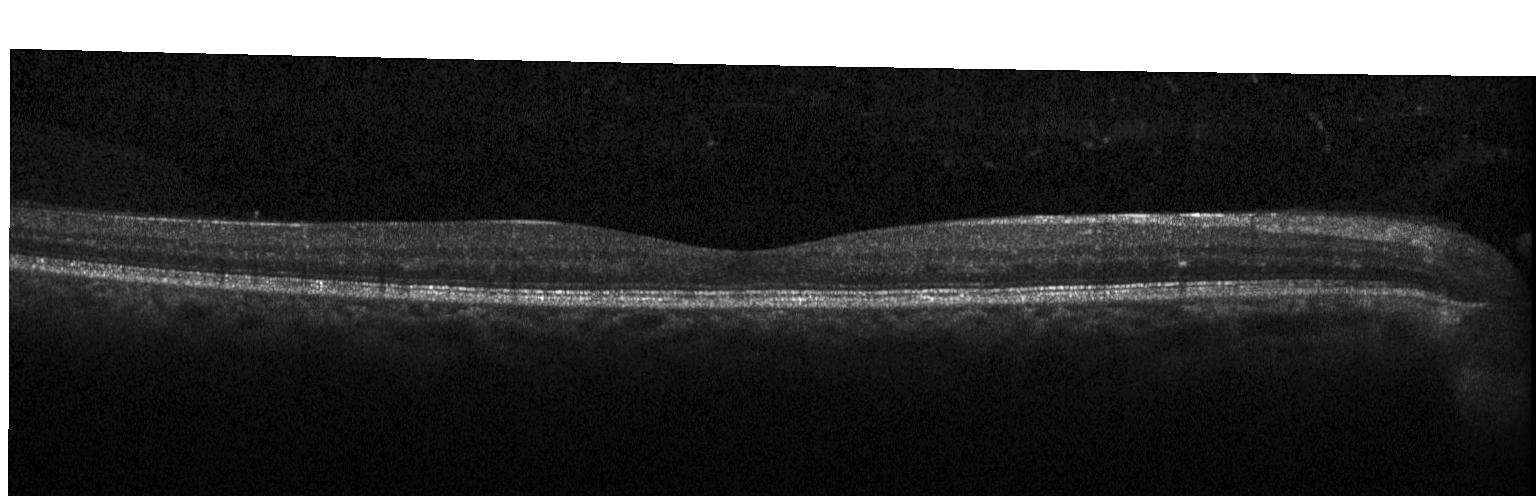
Horizontal scan through the fovea. Heidelberg Spectralis. Retinal OCT cross-section
The scan shows no choroidal neovascularization, diabetic macular edema, or drusen.